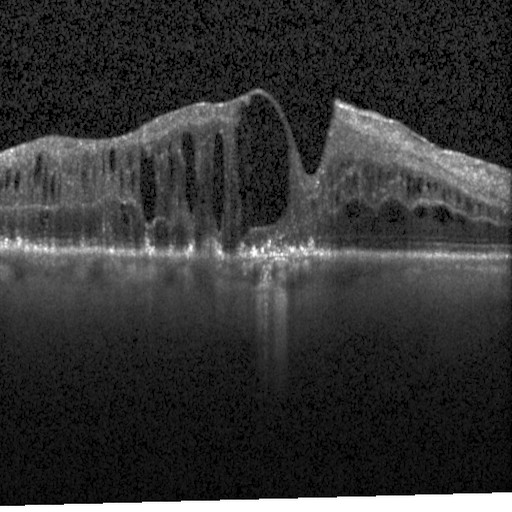 Optical coherence tomography B-scan — The scan shows diabetic macular edema.